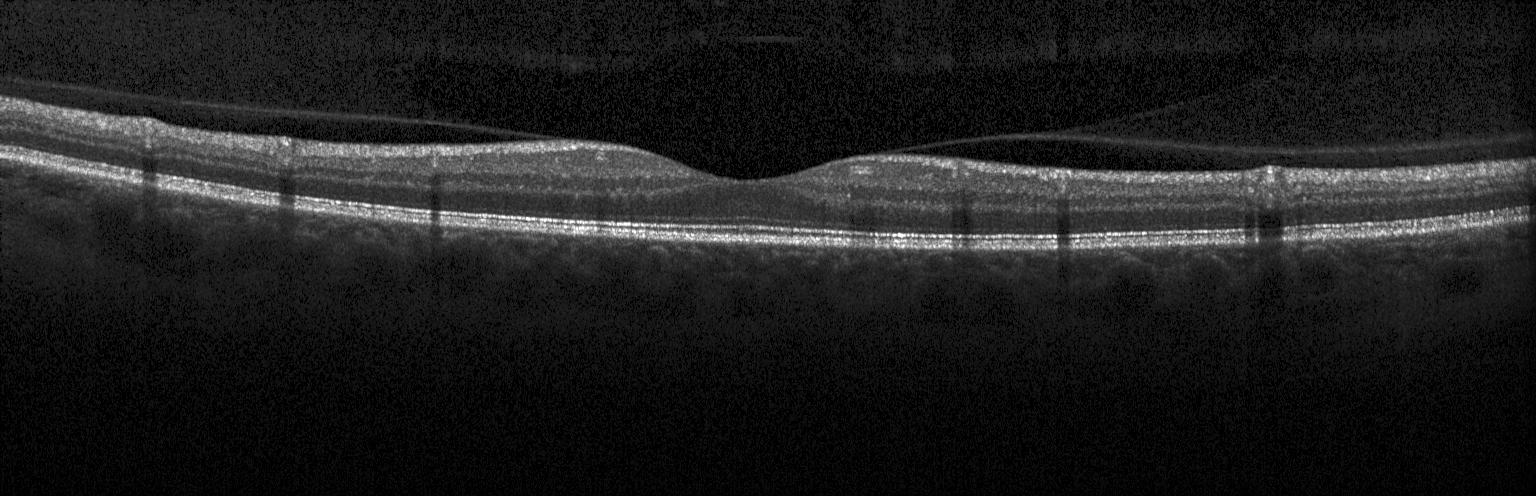 OCT line scan — Diagnosis: neither choroidal neovascularization, diabetic macular edema, nor drusen.